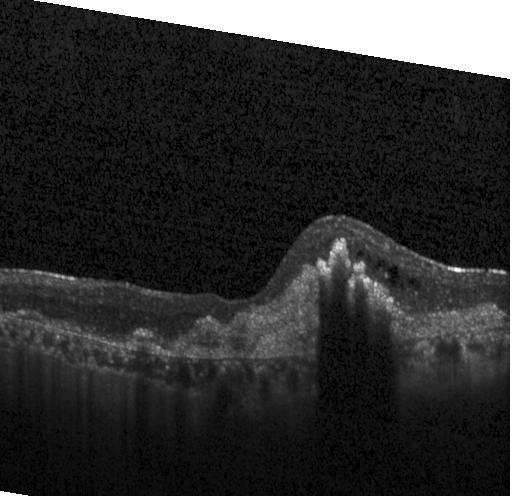
Spectral-domain optical coherence tomography; retinal OCT B-scan. Impression: choroidal neovascularization.